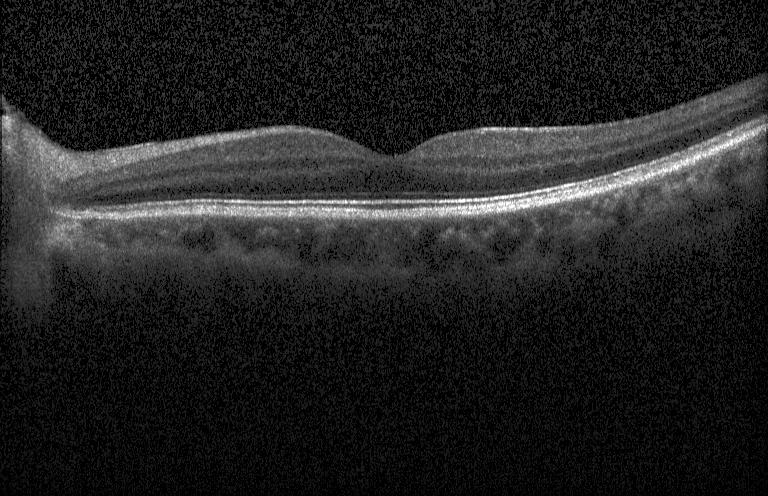
The scan shows no CNV, DME, or drusen.